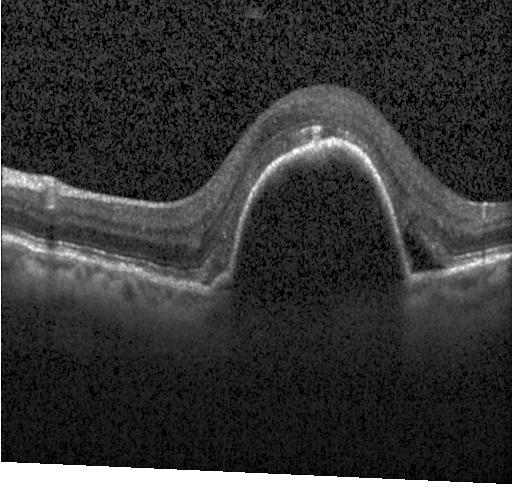

Retinal OCT cross-section showing choroidal neovascularization (CNV).